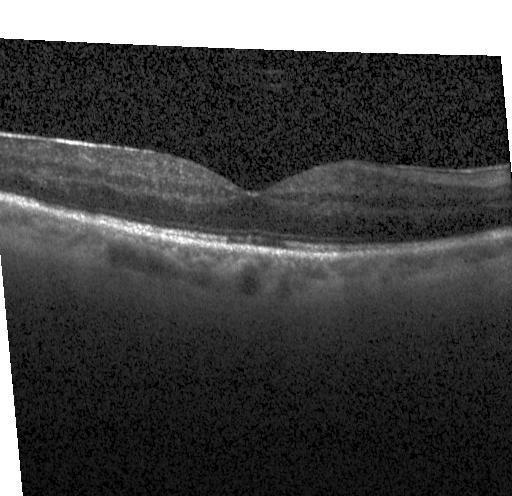 OCT B-scan. SD-OCT. Heidelberg Spectralis — Impression: neither choroidal neovascularization, diabetic macular edema, nor drusen.